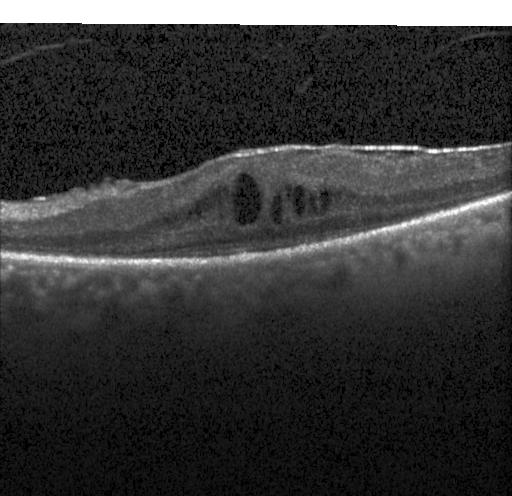 Macular OCT: diabetic macular edema (DME).